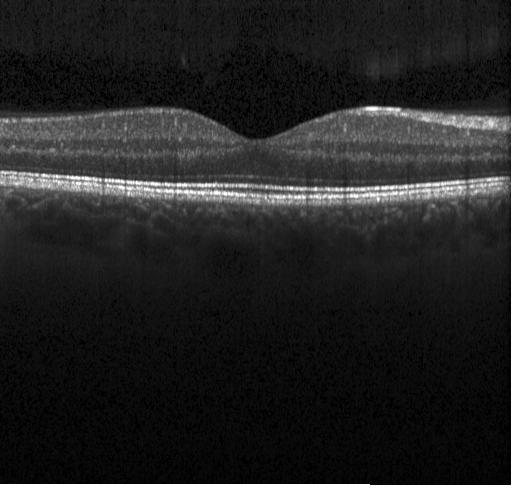

Spectral-domain optical coherence tomography · retinal OCT B-scan.
No evidence of choroidal neovascularization, diabetic macular edema, or drusen.